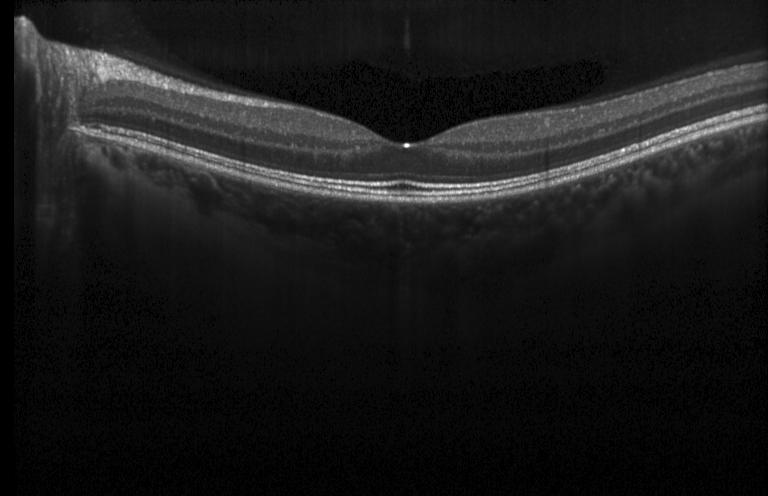 OCT line scan · spectral-domain optical coherence tomography. OCT finding: no choroidal neovascularization, diabetic macular edema, or drusen.